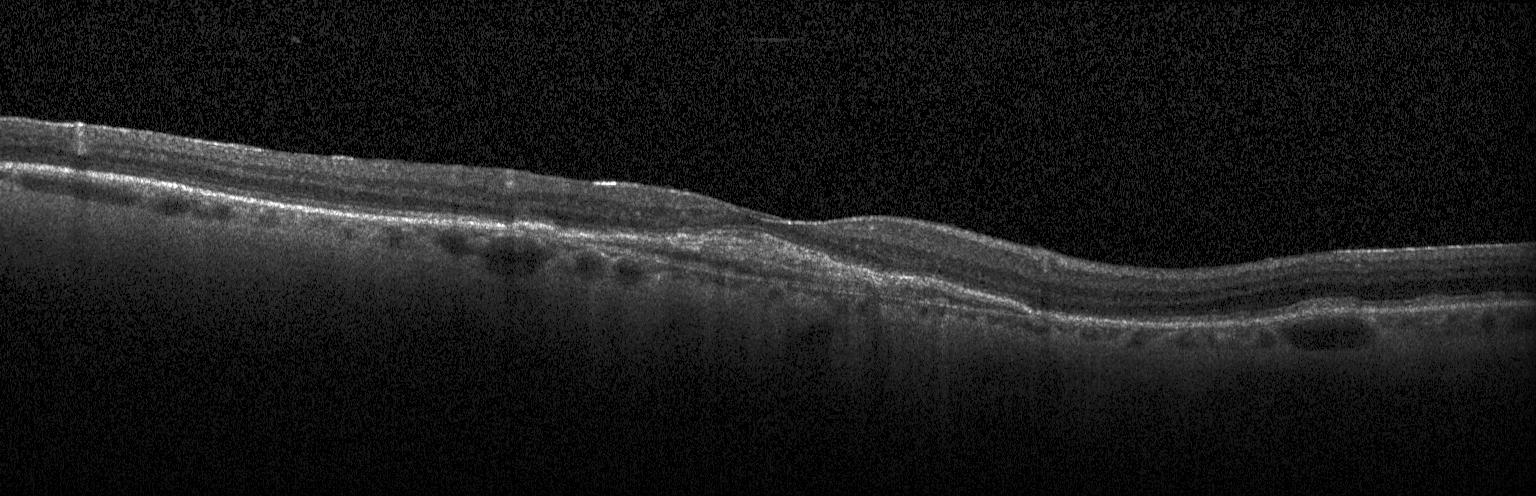
Diagnosis: choroidal neovascularization (CNV).